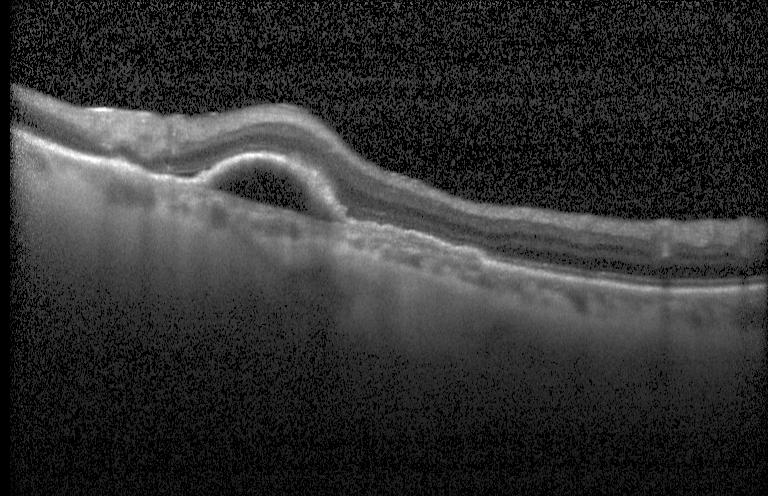 Assessment: a choroidal neovascular membrane.